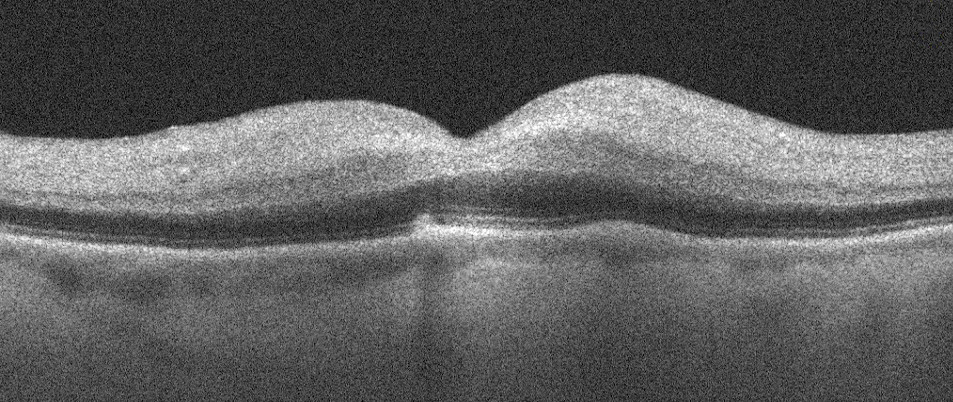 Macular scan, optical coherence tomography scan, instrument: Optovue Avanti RTVue XR. Impression: retinal artery occlusion.